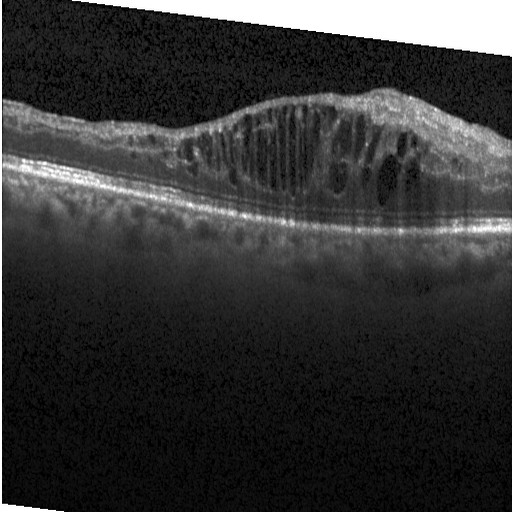
SD-OCT; optical coherence tomography scan
The scan shows DME.